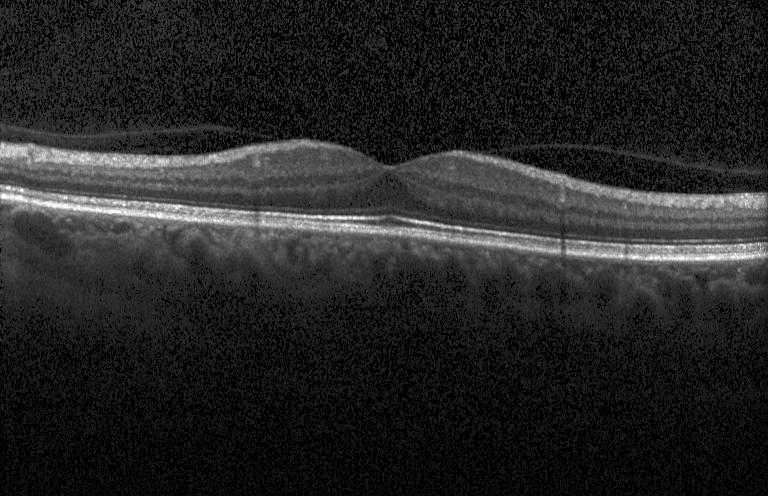
OCT B-scan showing no evidence of choroidal neovascularization, diabetic macular edema, or drusen.